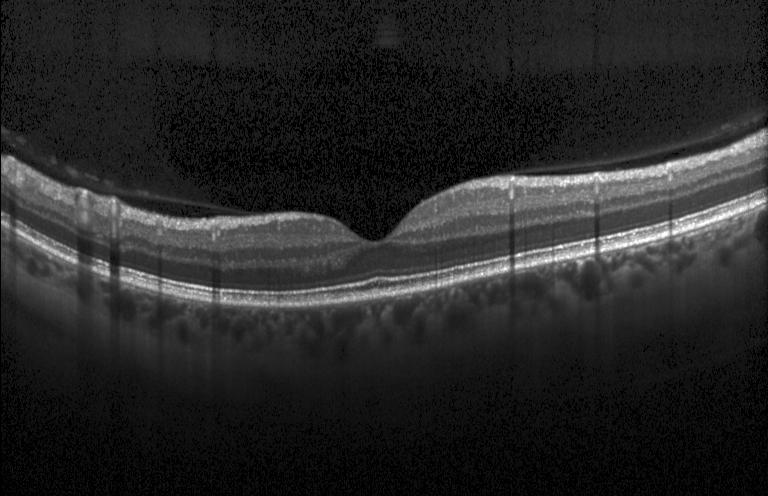
Finding: no CNV, DME, or drusen.